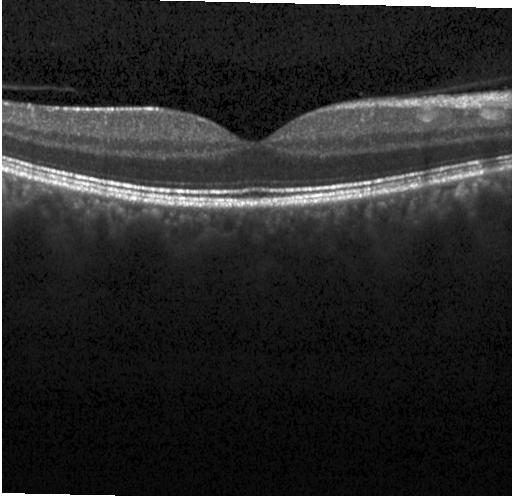 Fovea-centered; optical coherence tomography B-scan. Diagnosis: neither choroidal neovascularization, diabetic macular edema, nor drusen.